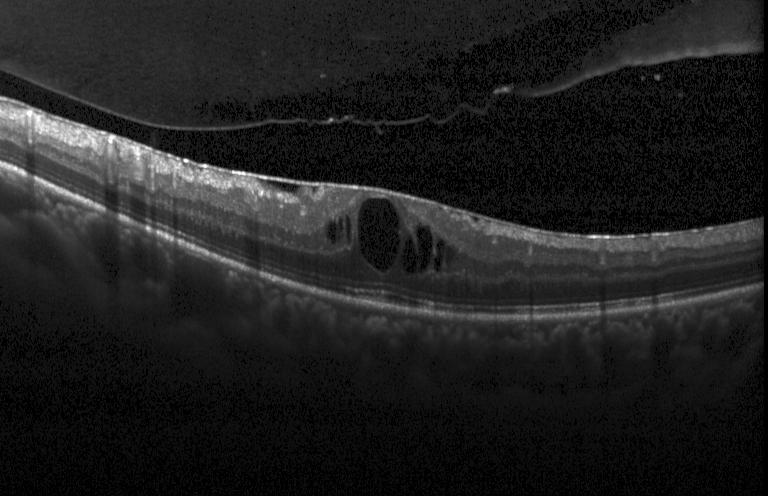 Retinal OCT cross-section
The scan shows diabetic macular edema.